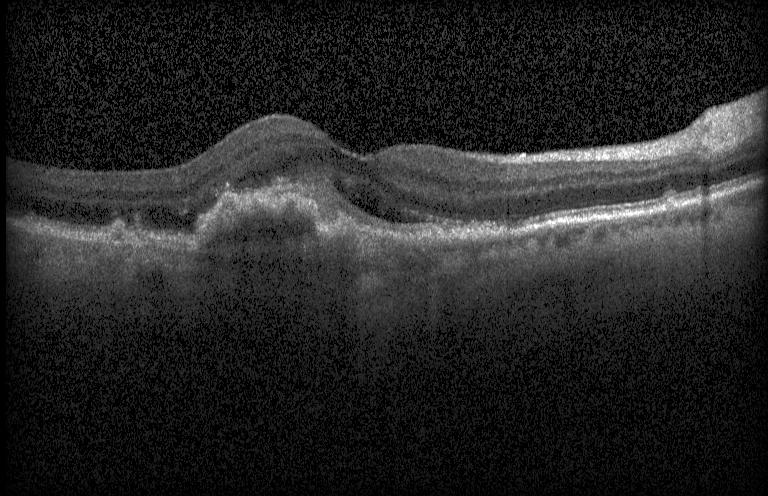
Diagnosis: a choroidal neovascular membrane.